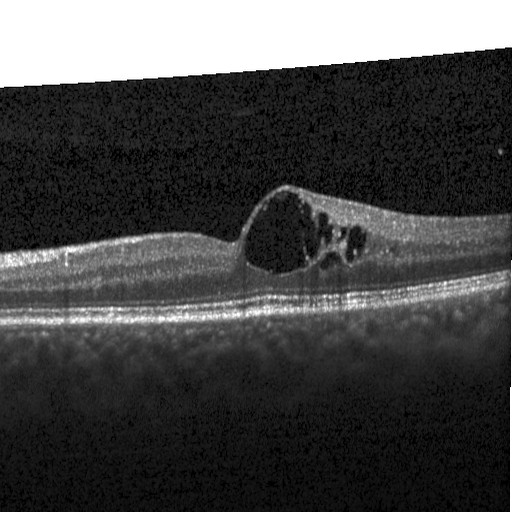
Optical coherence tomography B-scan; Heidelberg Spectralis; spectral-domain OCT; fovea-centered. OCT finding: DME.